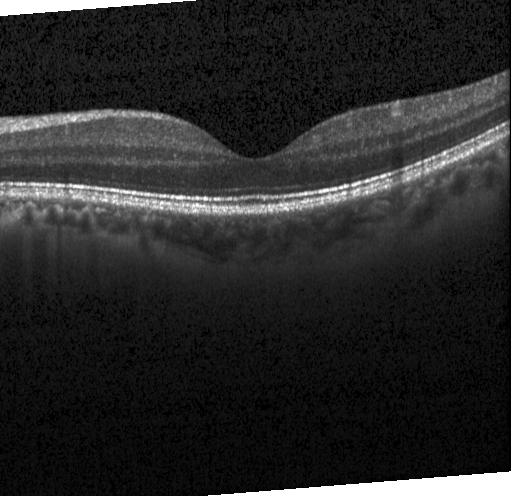 Finding: neither choroidal neovascularization, diabetic macular edema, nor drusen.